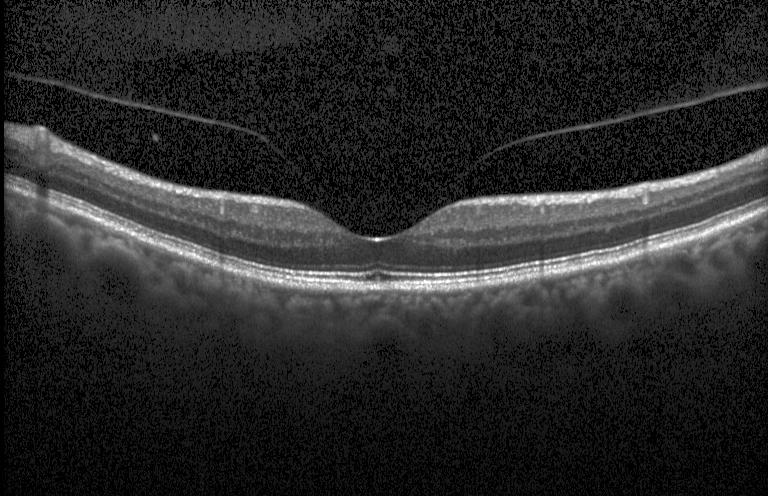
Retinal OCT cross-section
Diagnosis: no CNV, DME, or drusen.